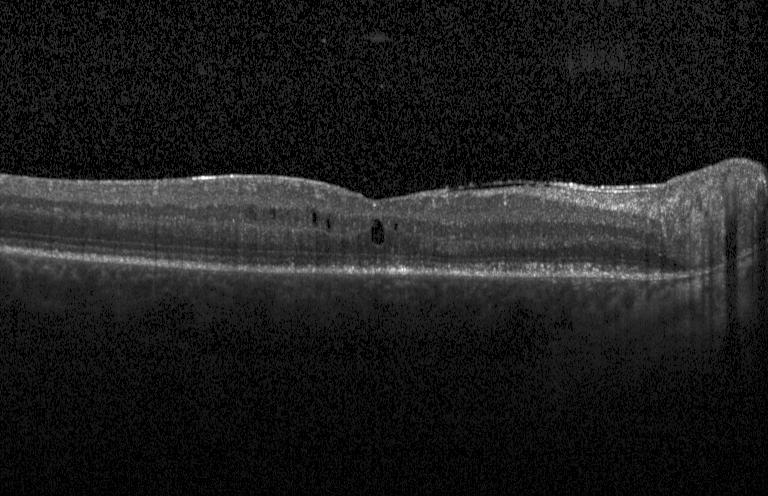

Assessment: diabetic macular edema (DME).